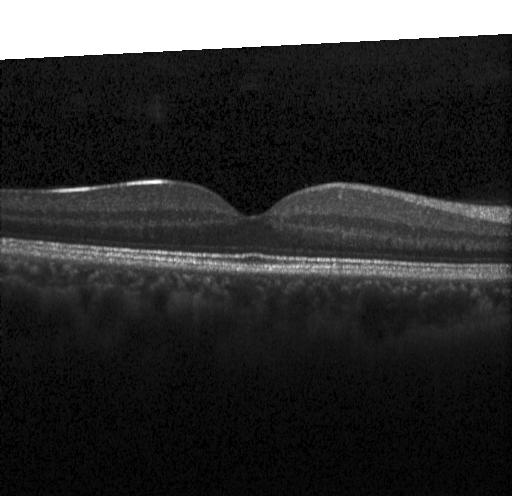

Optical coherence tomography scan
Finding: no choroidal neovascularization, diabetic macular edema, or drusen.